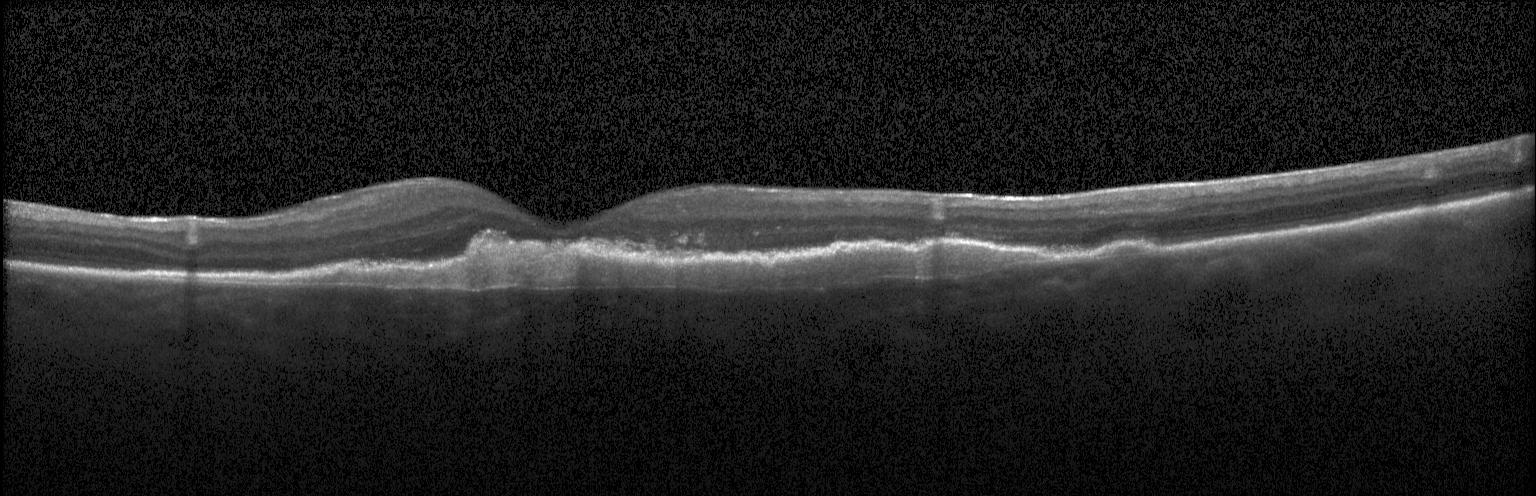
Through the macula. Instrument: Heidelberg Spectralis. Retinal OCT B-scan. Choroidal neovascularization (CNV).